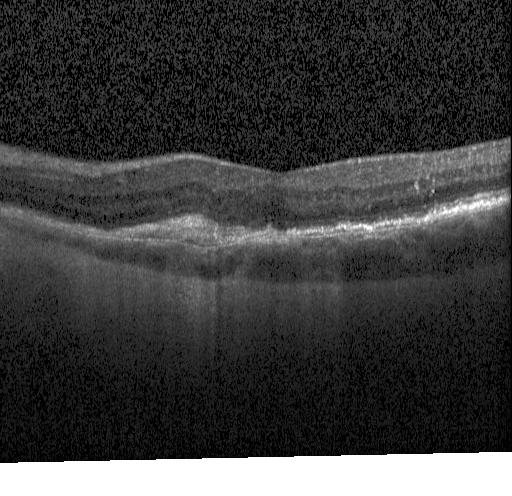 Horizontal scan through the fovea. Optical coherence tomography B-scan
Impression: choroidal neovascularization (CNV).